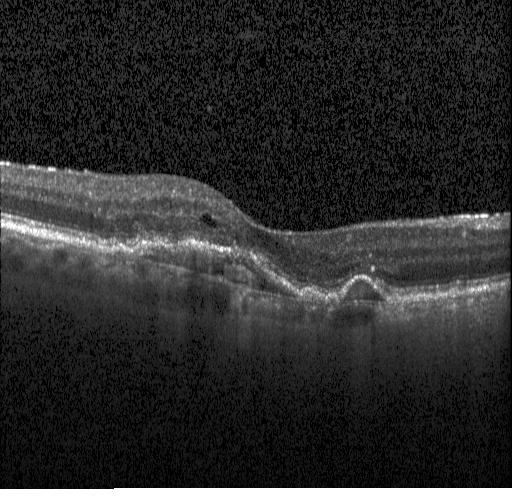

Finding: a choroidal neovascular membrane.